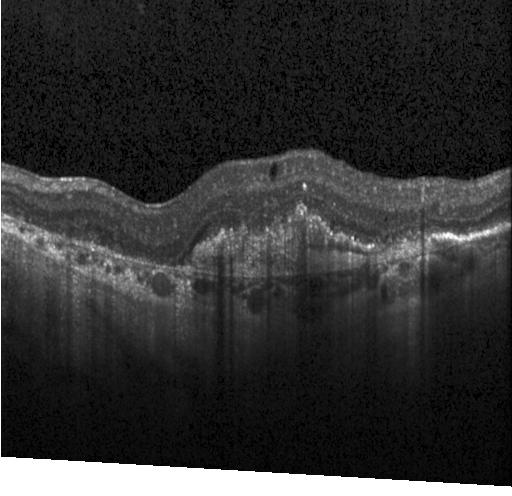
Diagnosis: a choroidal neovascular membrane.